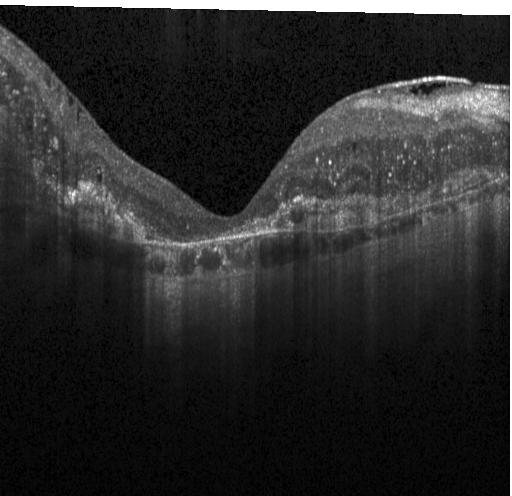
Optical coherence tomography B-scan · spectral-domain OCT · Heidelberg Spectralis · fovea-centered
OCT finding: a choroidal neovascular membrane.